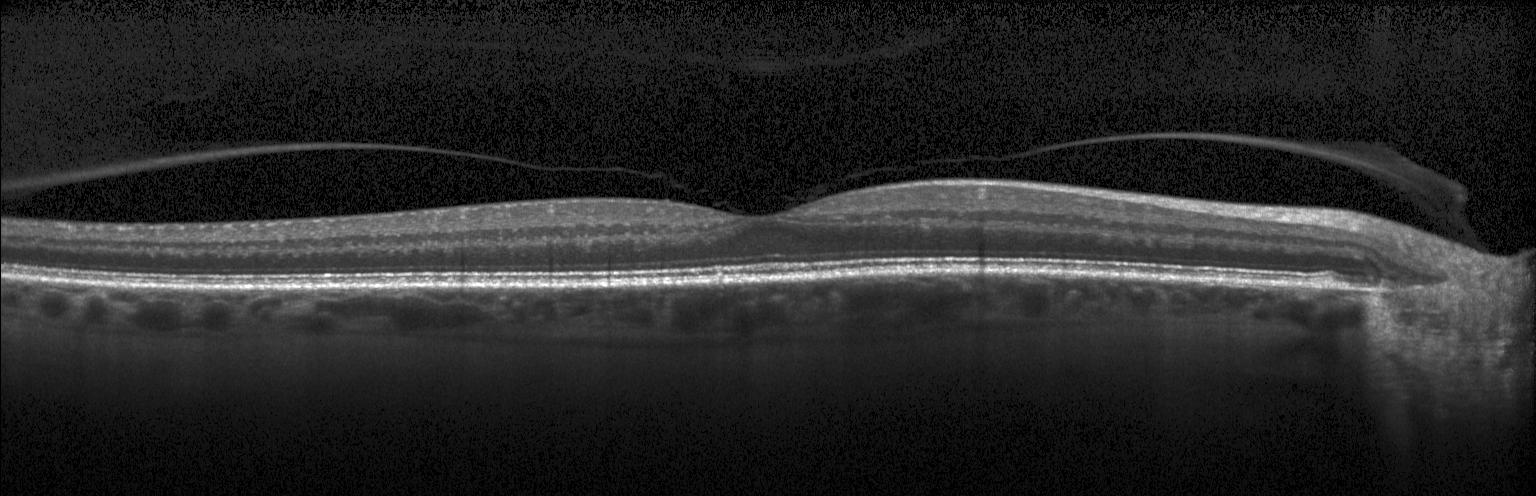

Finding: no choroidal neovascularization, diabetic macular edema, or drusen.